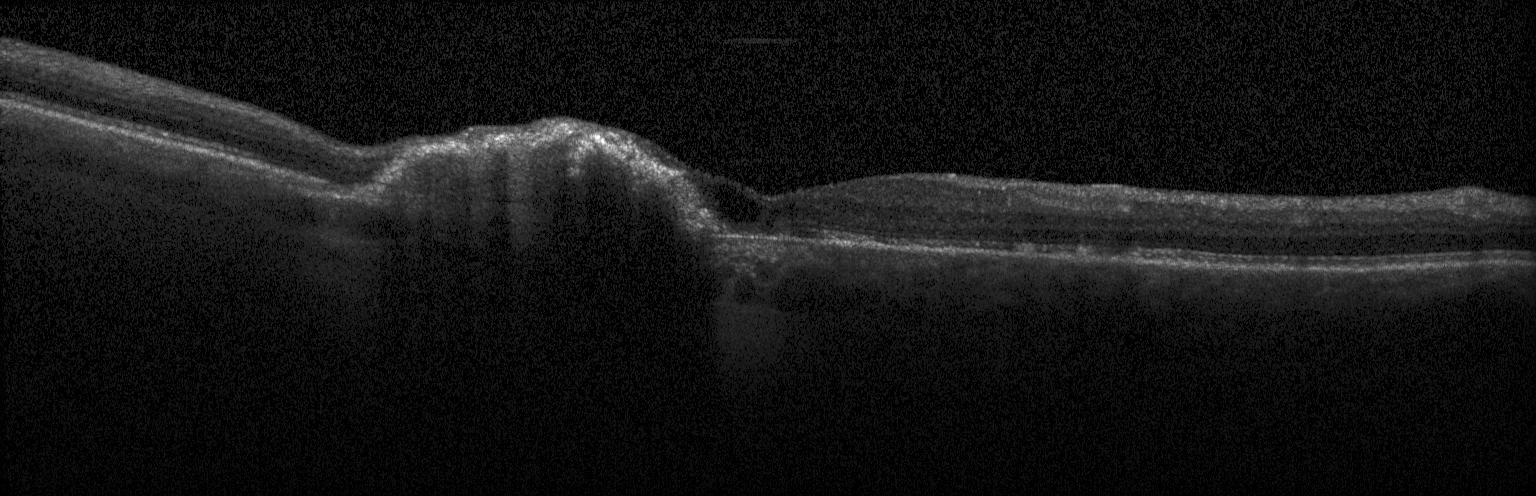

Optical coherence tomography B-scan; Heidelberg Spectralis OCT system.
Impression: choroidal neovascularization (CNV).